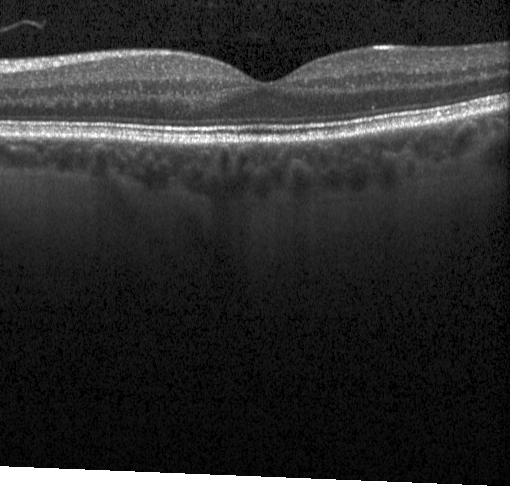 This B-scan demonstrates neither CNV, DME, nor drusen.